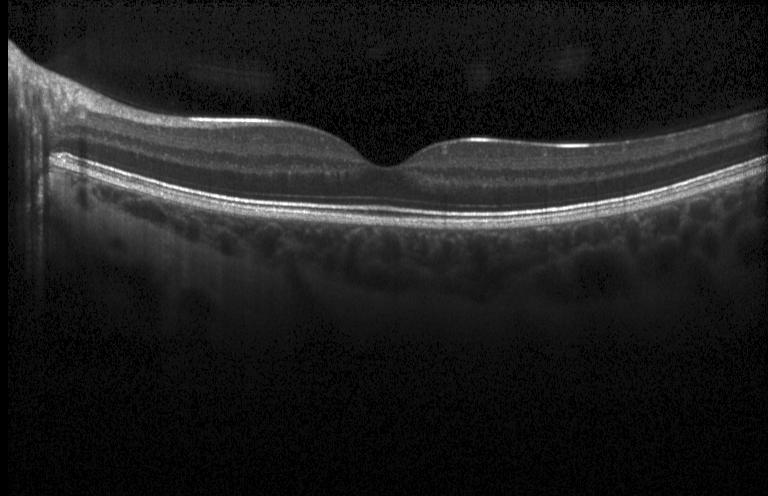
Optical coherence tomography B-scan; SD-OCT; acquired on a Heidelberg Spectralis — Finding: no choroidal neovascularization, diabetic macular edema, or drusen.